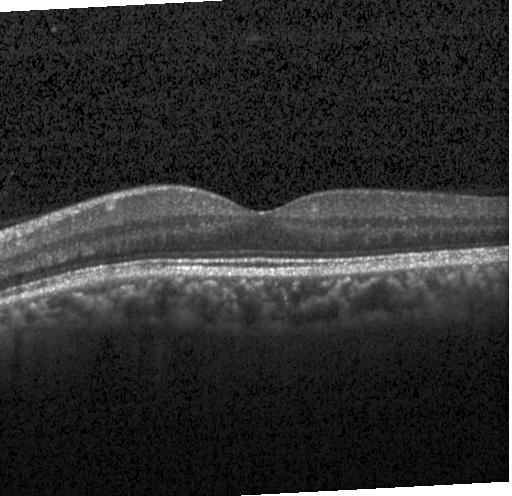 Macular scan, spectral-domain OCT, optical coherence tomography B-scan, instrument: Heidelberg Spectralis.
This B-scan demonstrates no choroidal neovascularization, no diabetic macular edema, and no drusen.